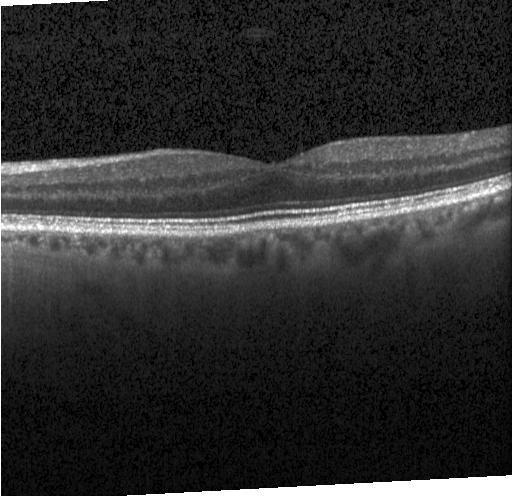
No choroidal neovascularization, diabetic macular edema, or drusen.